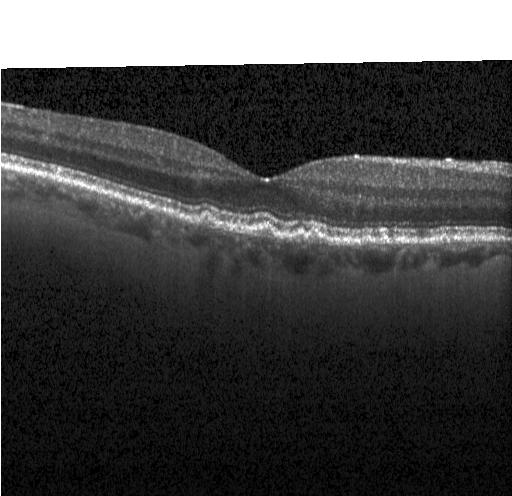

Heidelberg Spectralis OCT system, OCT B-scan, fovea-centered, spectral-domain optical coherence tomography. OCT finding: drusen.